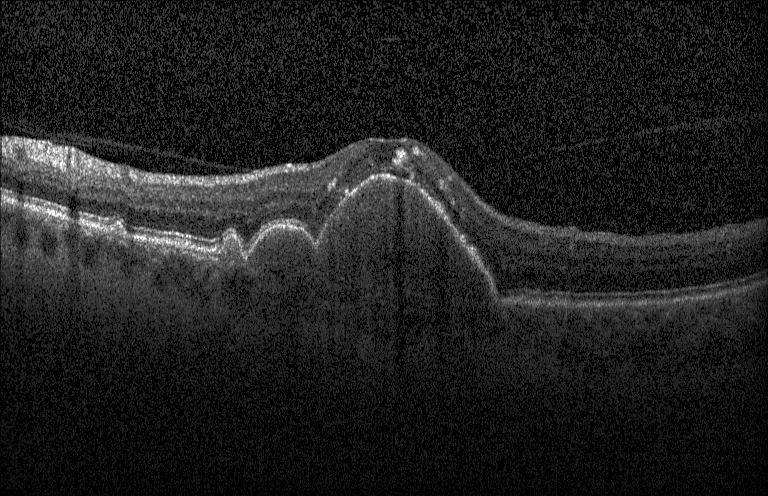

Optical coherence tomography scan · spectral-domain optical coherence tomography. The scan shows CNV.